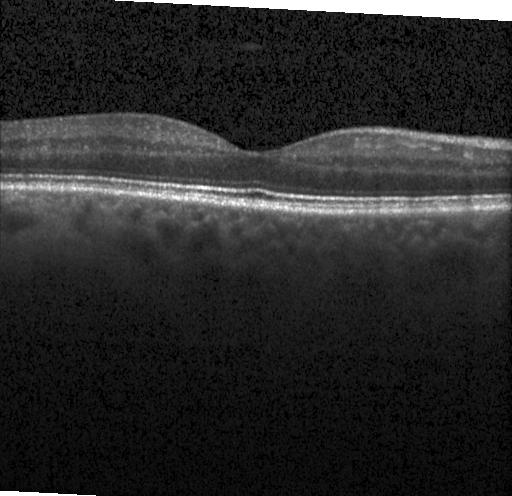

This B-scan demonstrates no choroidal neovascularization, no diabetic macular edema, and no drusen.